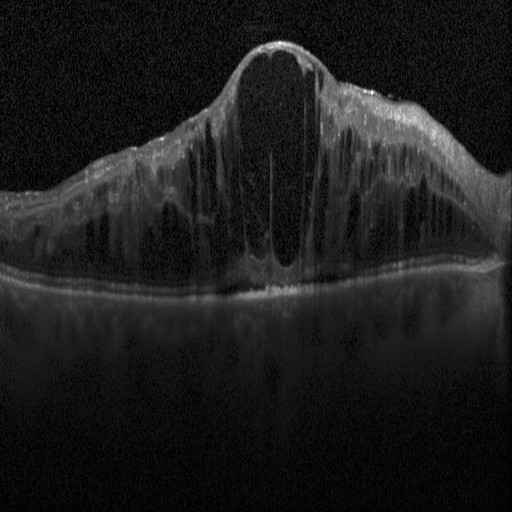

Diabetic macular edema (DME).